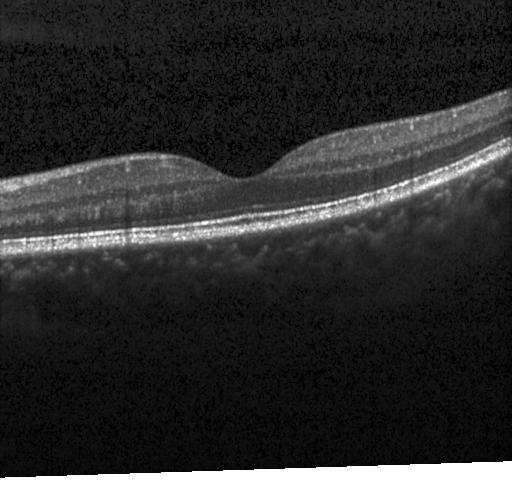

OCT line scan; macular scan; acquired on a Heidelberg Spectralis. OCT finding: no evidence of choroidal neovascularization, diabetic macular edema, or drusen.